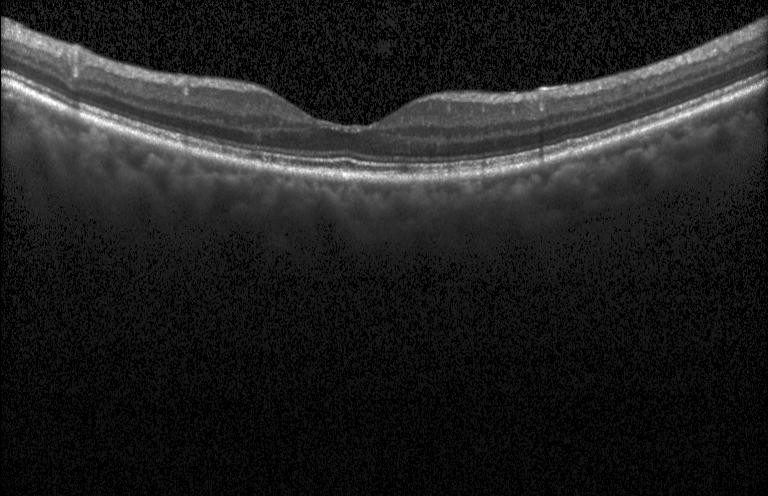

Retinal OCT cross-section; centered on the fovea — Impression: no evidence of choroidal neovascularization, diabetic macular edema, or drusen.